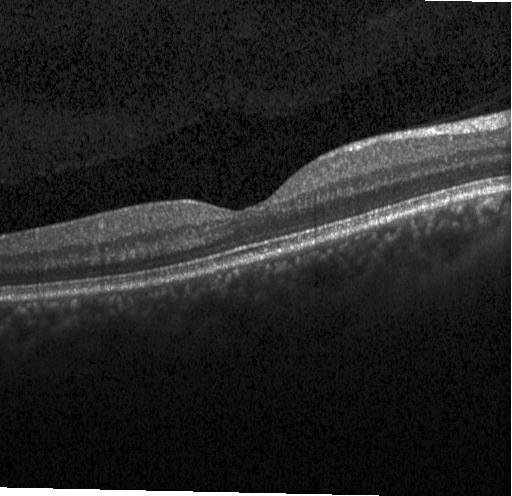

Spectral-domain optical coherence tomography; OCT B-scan; acquired on a Heidelberg Spectralis; fovea-centered — OCT finding: no CNV, DME, or drusen.